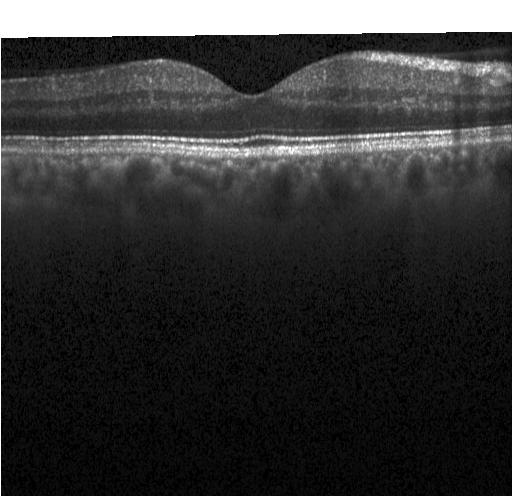

Horizontal scan through the fovea · retinal OCT cross-section.
Diagnosis: no choroidal neovascularization, no diabetic macular edema, and no drusen.